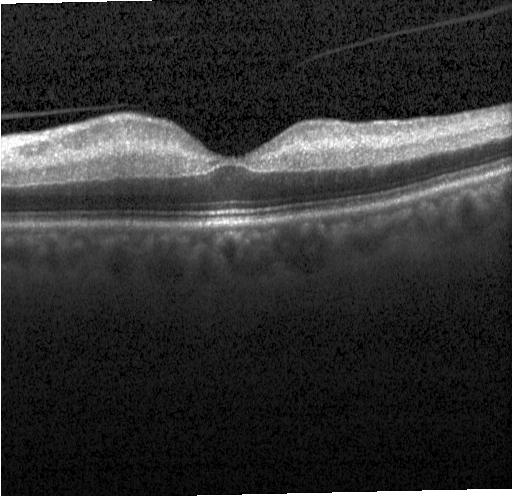
OCT finding: no choroidal neovascularization, diabetic macular edema, or drusen.